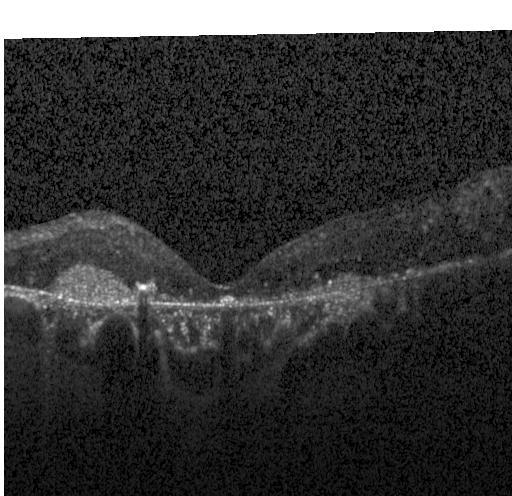 Through the macula, retinal OCT cross-section. Finding: a choroidal neovascular membrane.